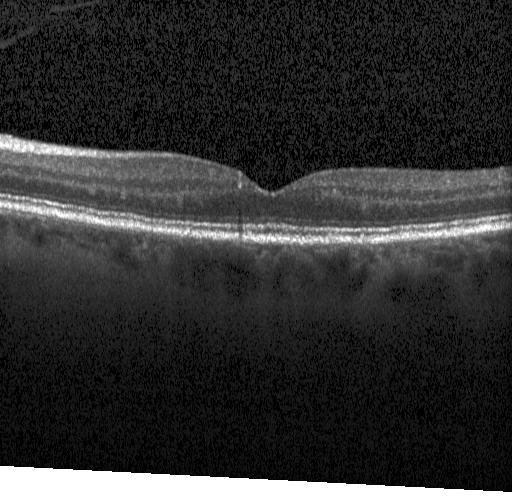 Centered on the fovea · optical coherence tomography B-scan.
This B-scan demonstrates no choroidal neovascularization, diabetic macular edema, or drusen.